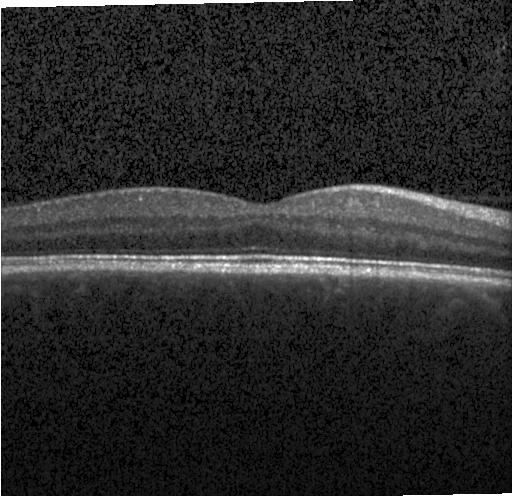 Macular scan; optical coherence tomography B-scan; instrument: Heidelberg Spectralis; spectral-domain OCT.
Finding: neither choroidal neovascularization, diabetic macular edema, nor drusen.